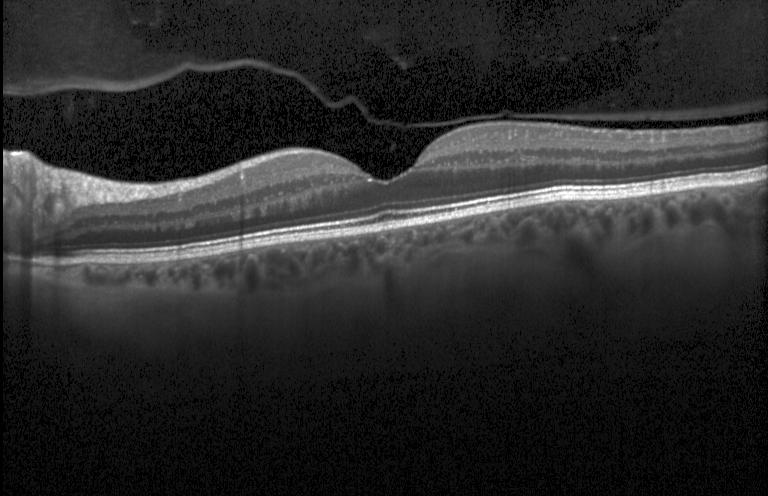 OCT line scan; Heidelberg Spectralis OCT system; through the macula — Assessment: no choroidal neovascularization, no diabetic macular edema, and no drusen.